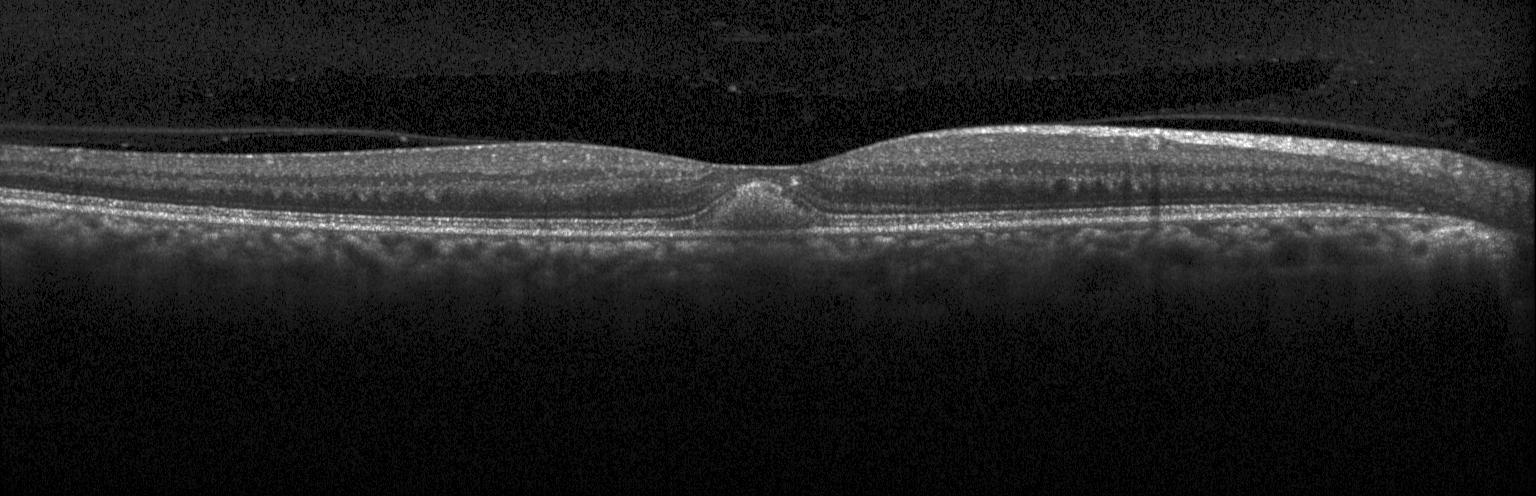
Spectral-domain optical coherence tomography, acquired on a Heidelberg Spectralis, centered on the fovea, OCT B-scan — Diagnosis: a choroidal neovascular membrane.